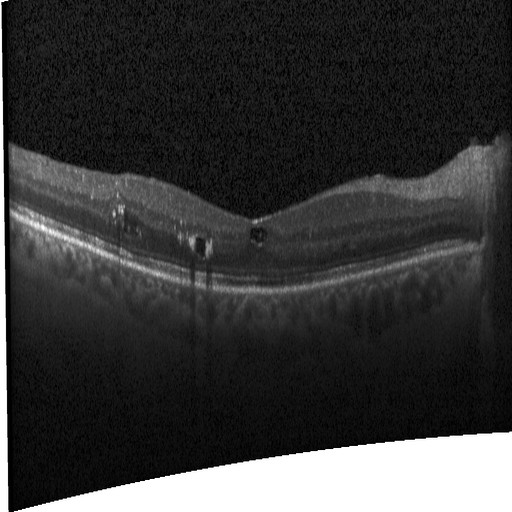 Impression: diabetic macular edema.